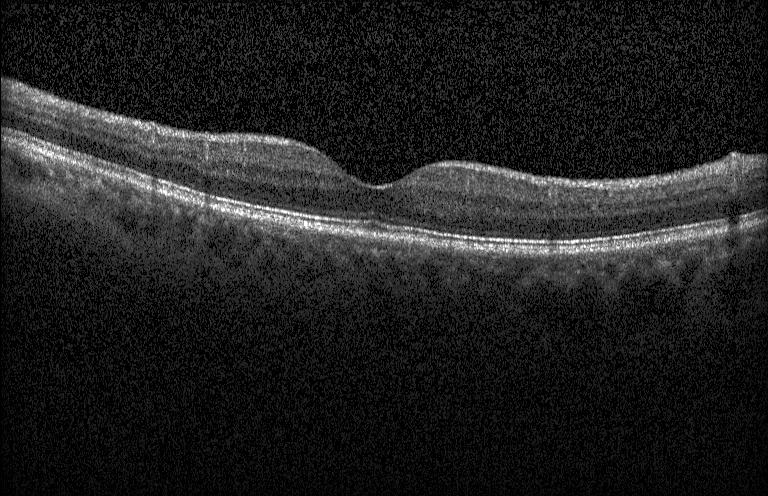

Finding: no evidence of choroidal neovascularization, diabetic macular edema, or drusen.